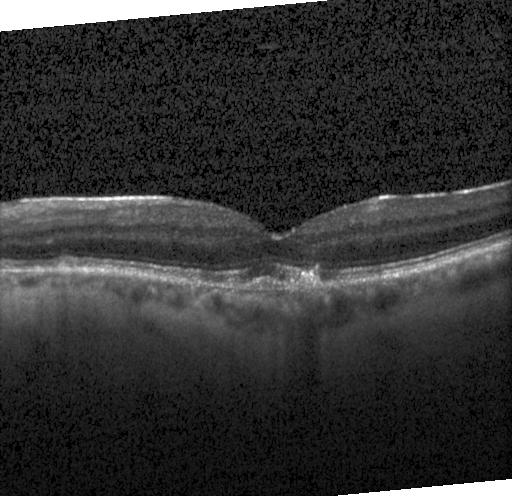
SD-OCT · optical coherence tomography scan · centered on the fovea · Heidelberg Spectralis OCT system.
CNV.